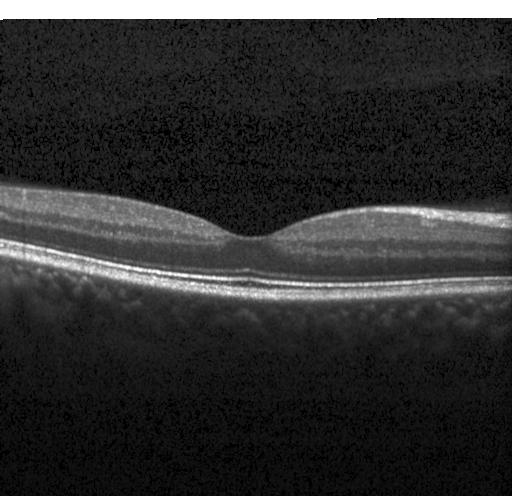

No evidence of CNV, DME, or drusen.